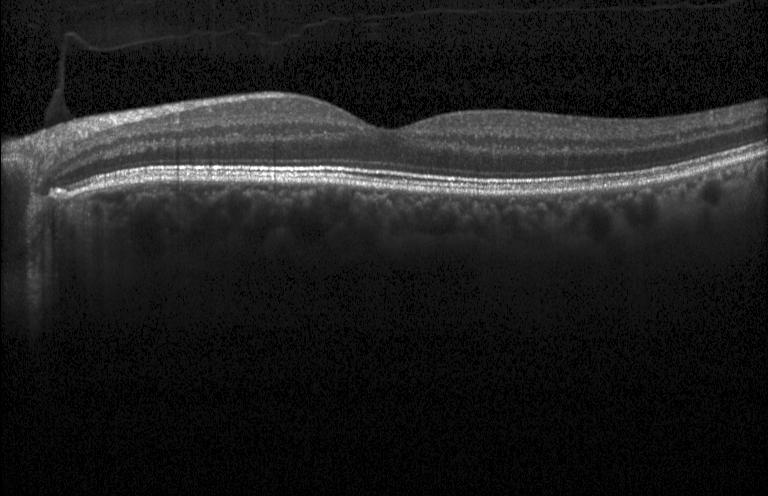 Optical coherence tomography scan. Assessment: no choroidal neovascularization, diabetic macular edema, or drusen.